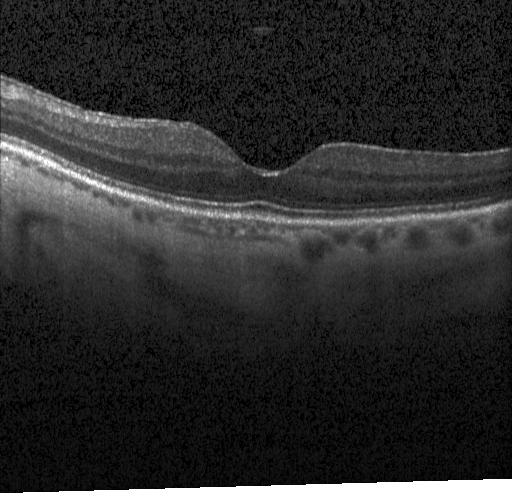 Retinal OCT cross-section showing no choroidal neovascularization, diabetic macular edema, or drusen.